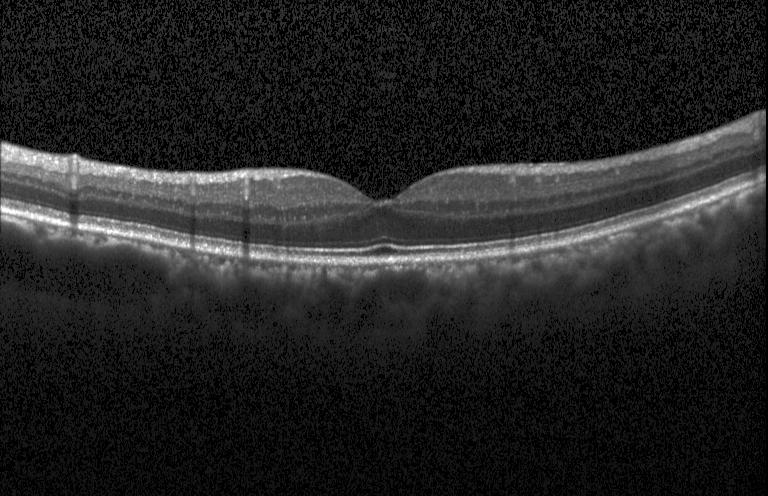

Horizontal scan through the fovea · instrument: Heidelberg Spectralis · OCT line scan · spectral-domain optical coherence tomography
Macular OCT: neither CNV, DME, nor drusen.